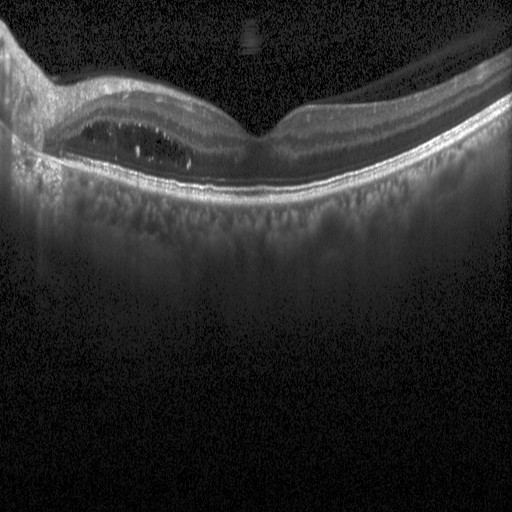
OCT line scan. Finding: diabetic macular edema (DME).